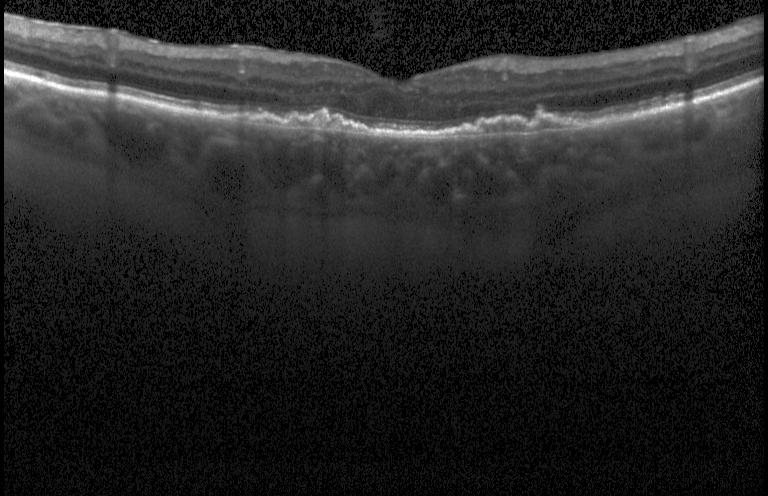
Diagnosis: a choroidal neovascular membrane.